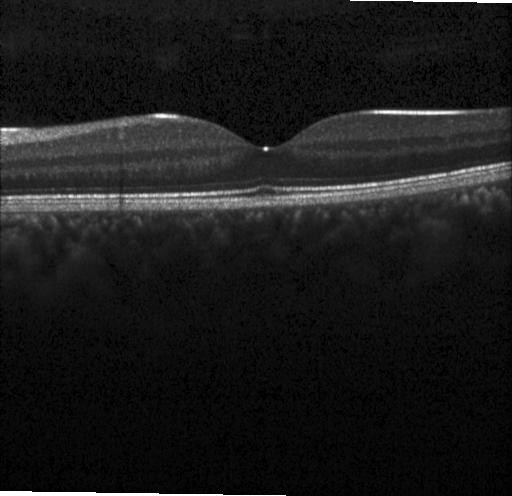
OCT line scan — Finding: no choroidal neovascularization, diabetic macular edema, or drusen.